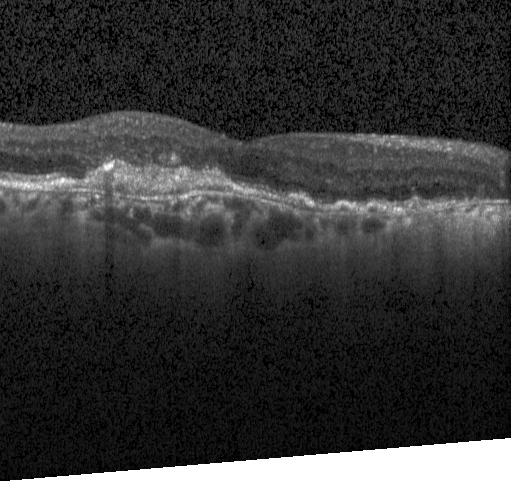

Macular OCT: CNV.